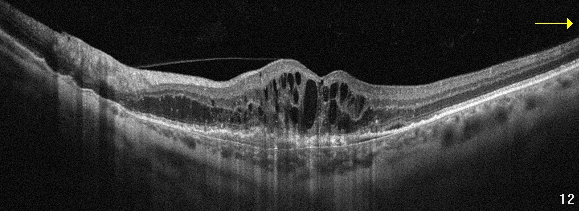
Optical coherence tomography scan; fovea-centered.
Macular OCT: age-related macular degeneration.